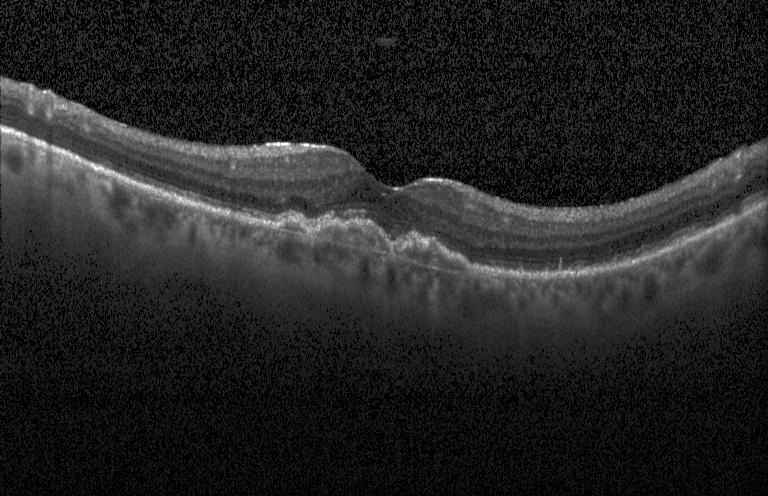
OCT finding: a choroidal neovascular membrane.